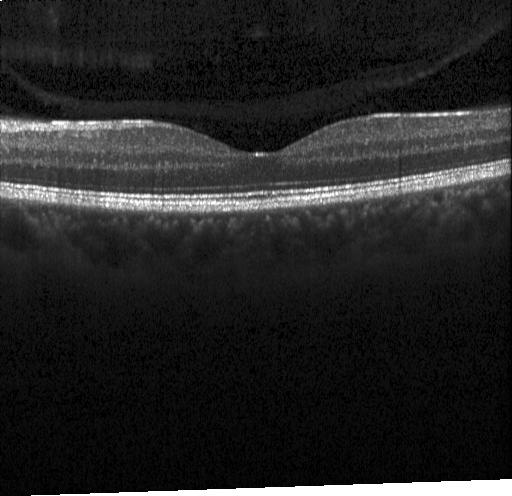
Retinal OCT cross-section showing no CNV, DME, or drusen.